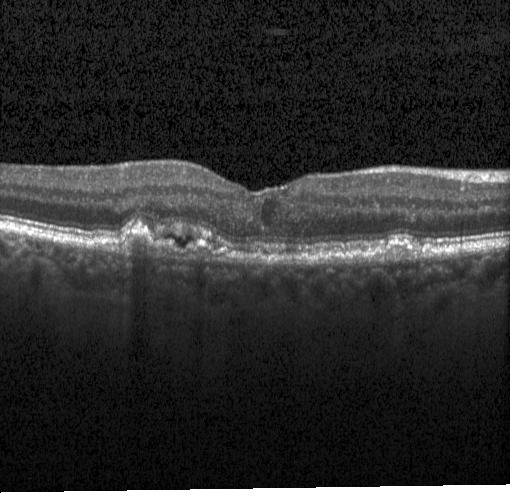 OCT B-scan showing choroidal neovascularization (CNV).